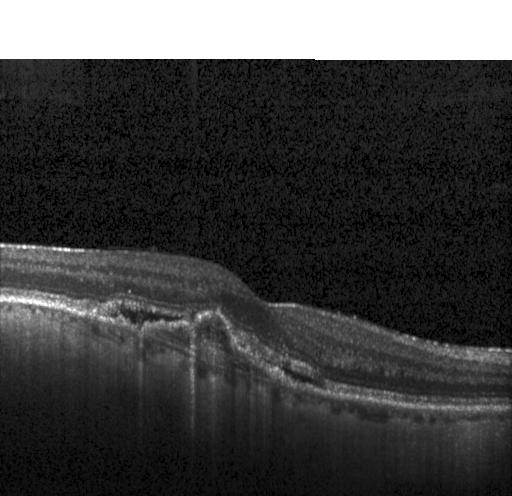

OCT B-scan. Impression: a choroidal neovascular membrane.